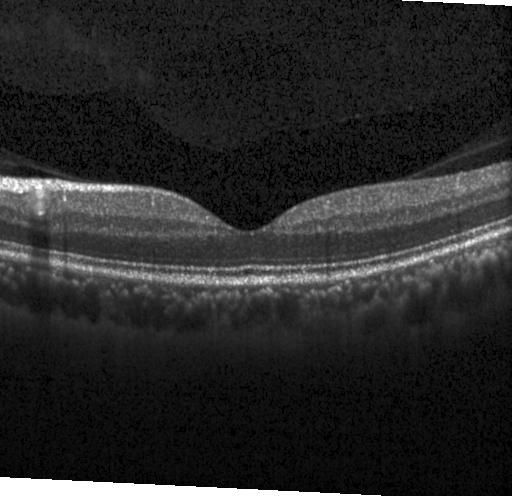

Spectral-domain OCT B-scan: neither choroidal neovascularization, diabetic macular edema, nor drusen.